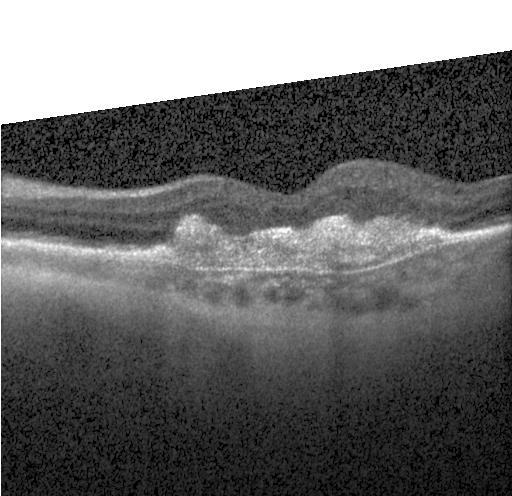
SD-OCT, Heidelberg Spectralis OCT system, retinal OCT B-scan.
OCT finding: CNV.